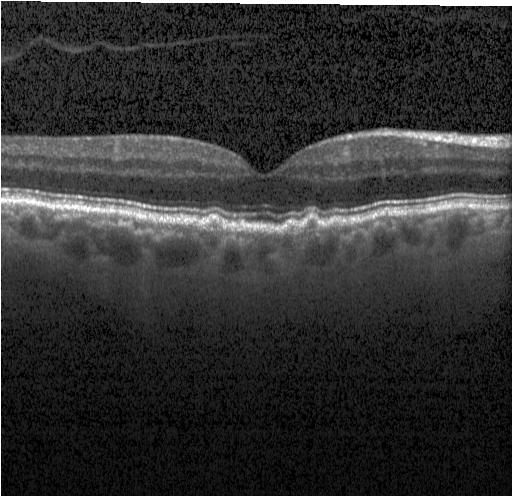 Spectral-domain optical coherence tomography · optical coherence tomography scan
The scan shows multiple drusen.